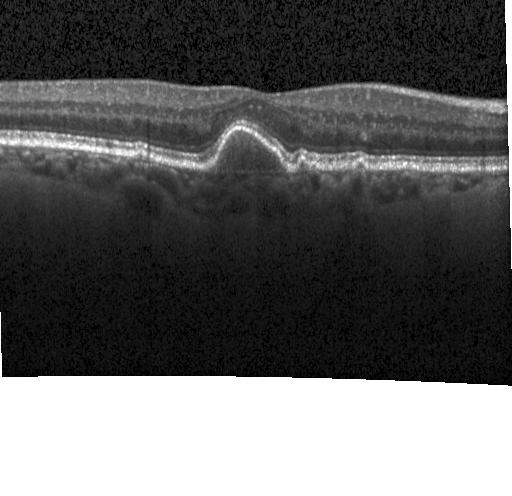
Retinal OCT B-scan. Macular OCT: a choroidal neovascular membrane.